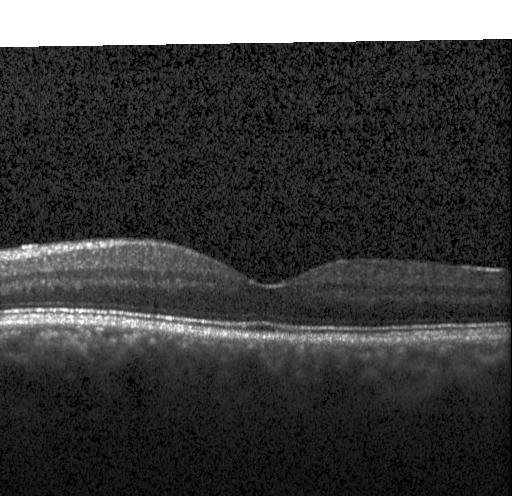
Diagnosis: no evidence of choroidal neovascularization, diabetic macular edema, or drusen.